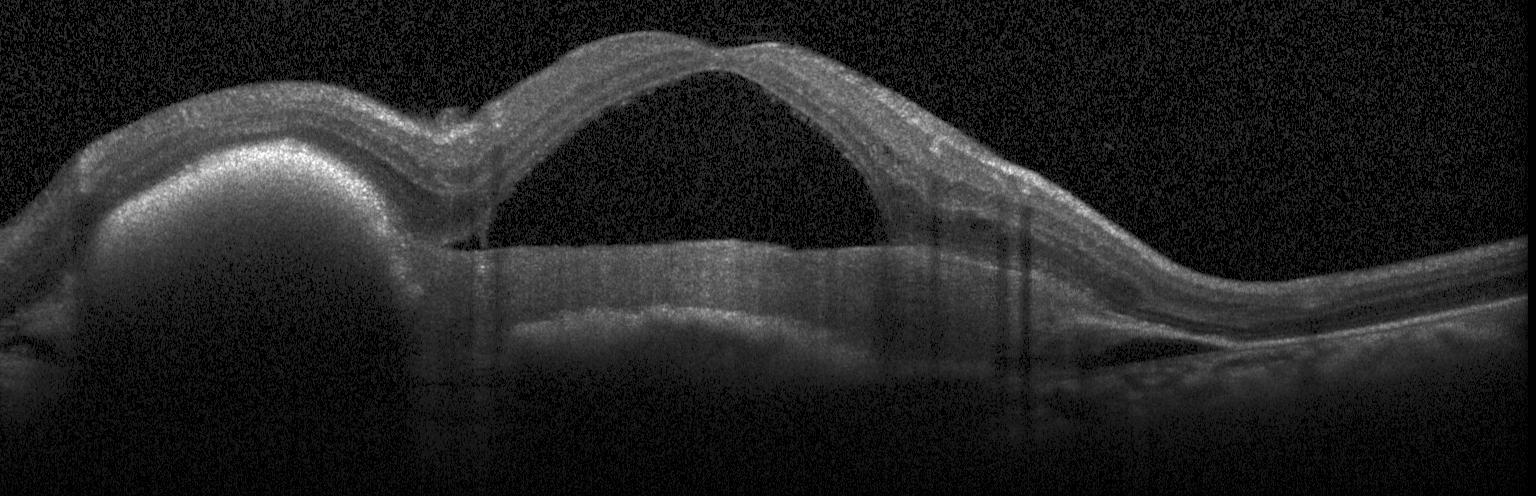 Macular scan · OCT line scan.
A choroidal neovascular membrane.